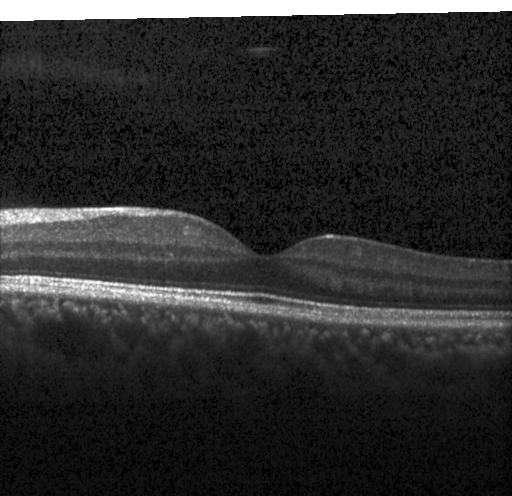
Assessment: no choroidal neovascularization, no diabetic macular edema, and no drusen.